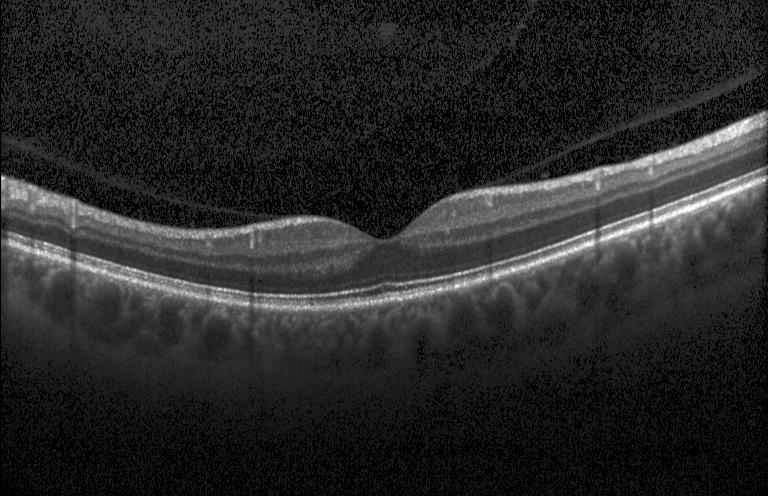 Retinal OCT B-scan. Finding: no evidence of choroidal neovascularization, diabetic macular edema, or drusen.